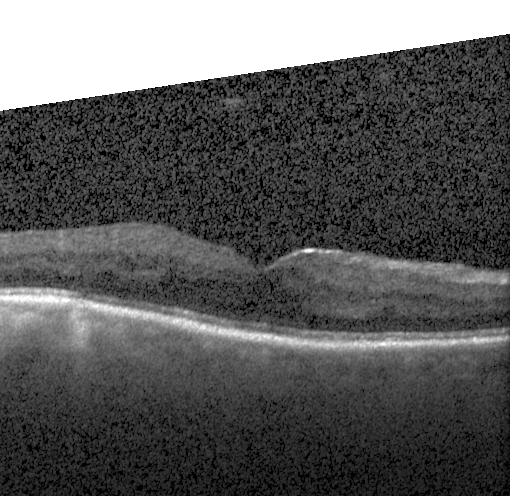

Finding: no evidence of choroidal neovascularization, diabetic macular edema, or drusen.